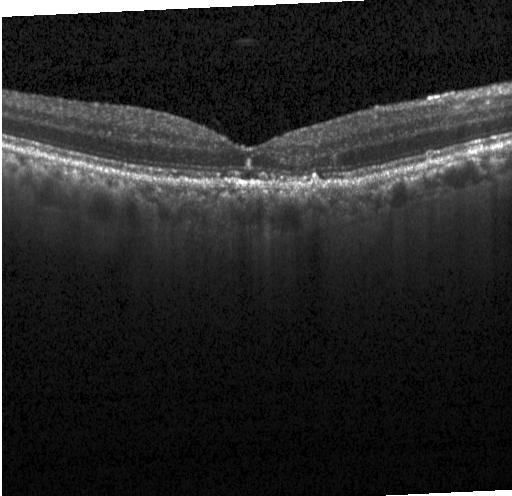

This B-scan demonstrates sub-RPE drusenoid deposits.